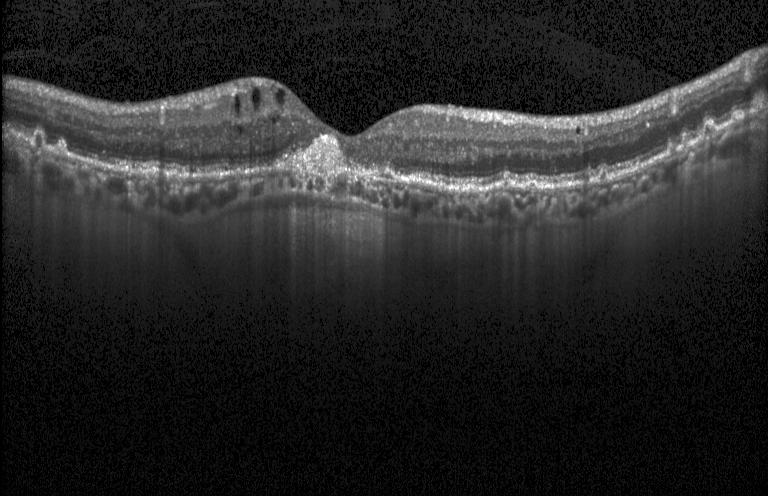

OCT B-scan. SD-OCT.
OCT finding: choroidal neovascularization.